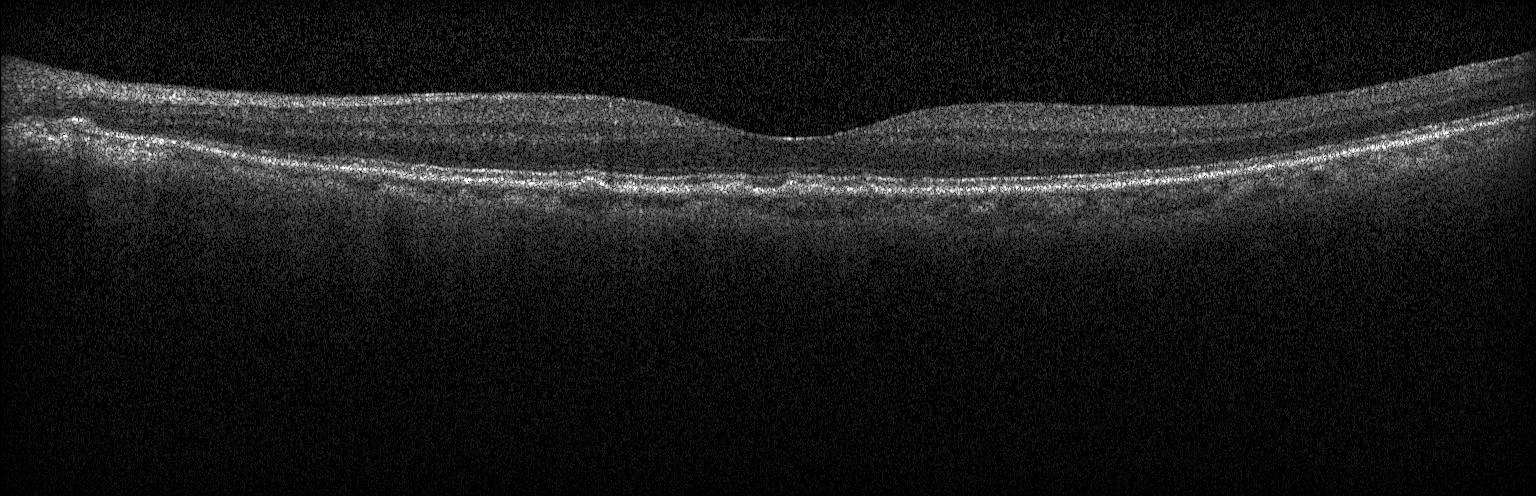

Optical coherence tomography scan, through the macula.
Finding: sub-RPE drusenoid deposits.